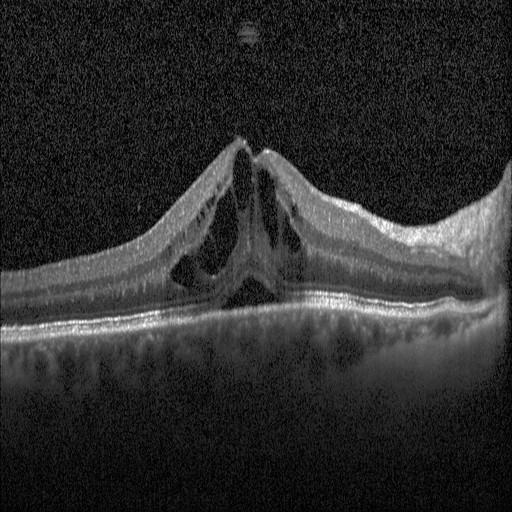

Assessment: diabetic macular edema.